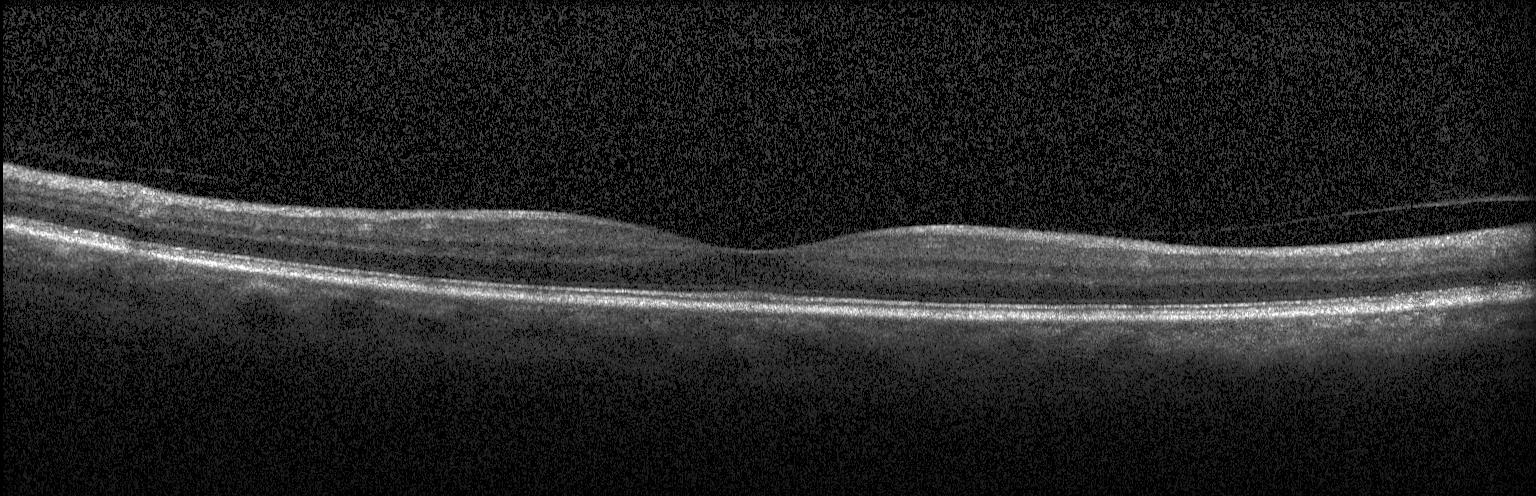 Optical coherence tomography scan. Through the macula.
Assessment: no choroidal neovascularization, no diabetic macular edema, and no drusen.